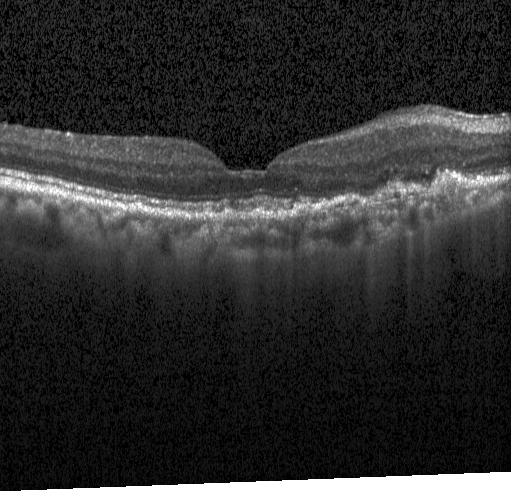

Dx: CNV.